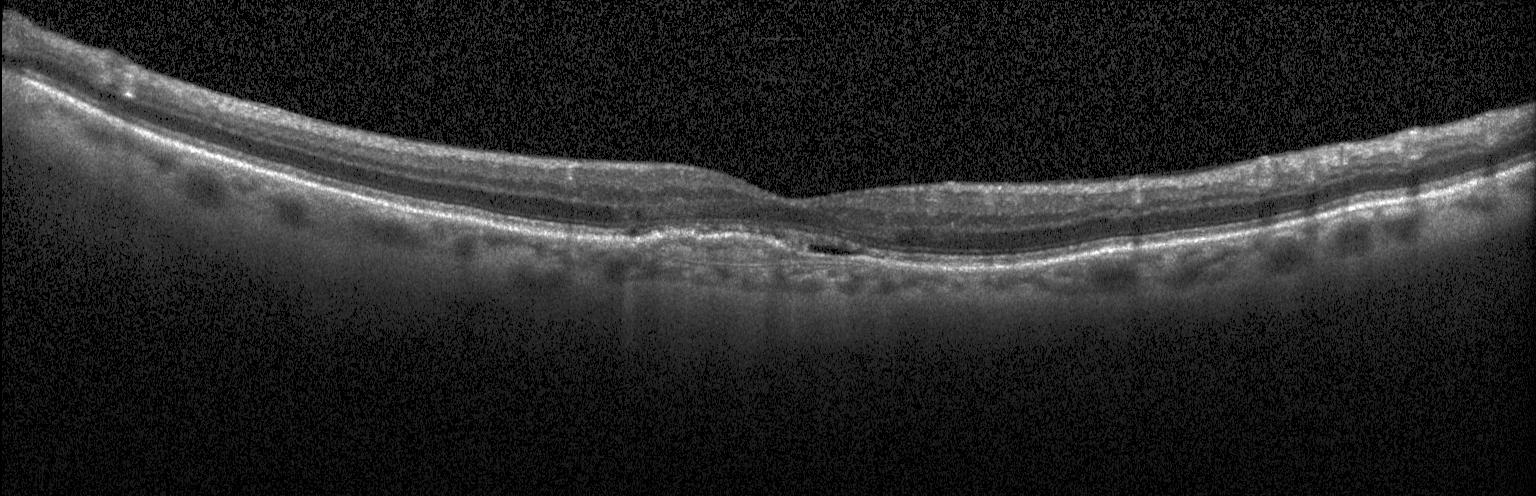
OCT finding: choroidal neovascularization.